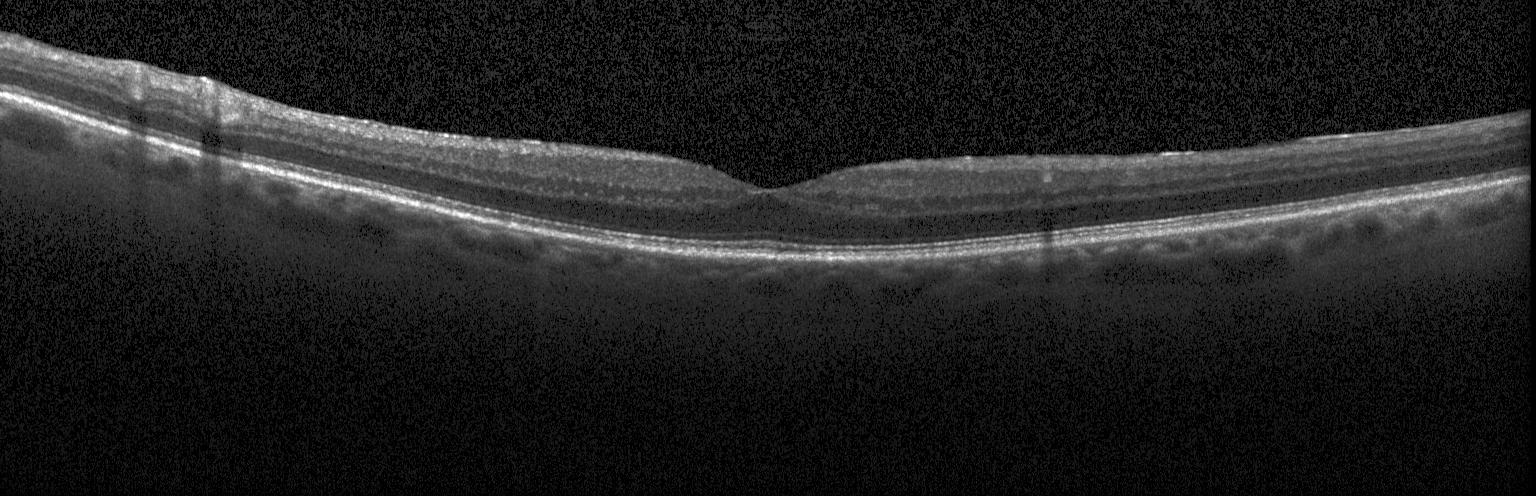 Diagnosis: no CNV, no DME, and no drusen.